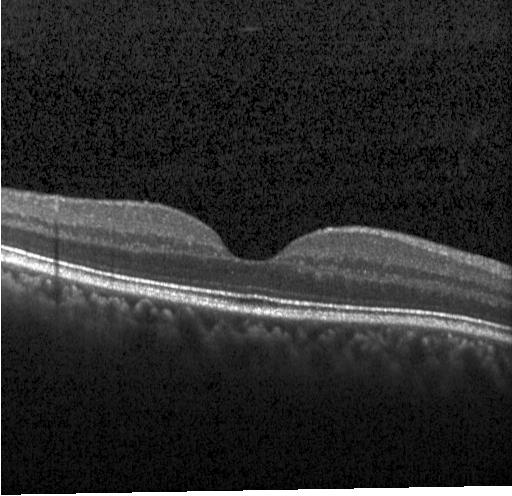

OCT finding: no choroidal neovascularization, diabetic macular edema, or drusen.